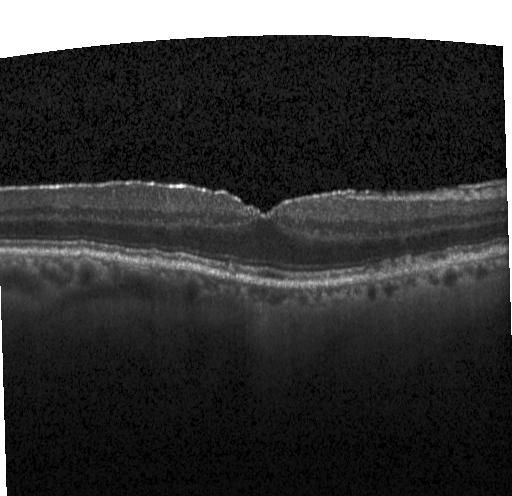 Impression: multiple drusen.